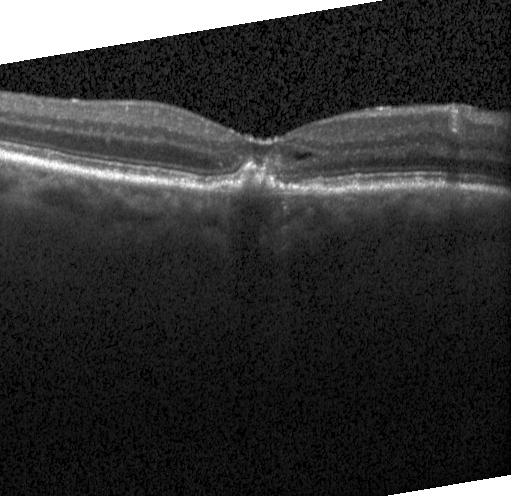
Retinal OCT B-scan
Dx: a choroidal neovascular membrane.